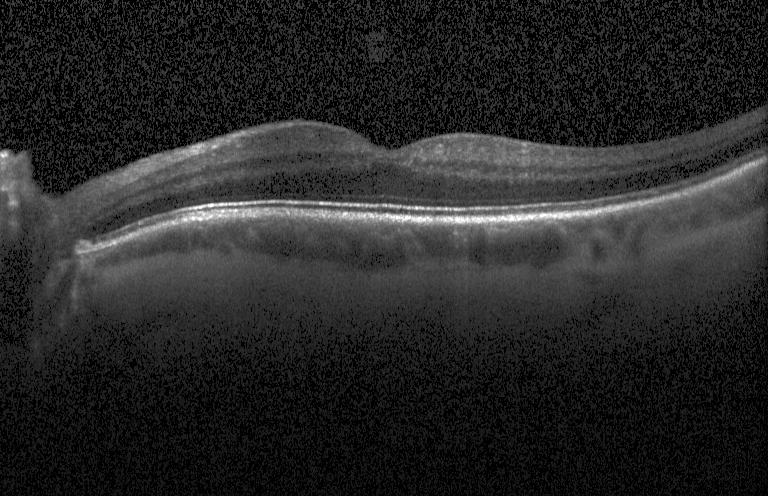 Impression: neither choroidal neovascularization, diabetic macular edema, nor drusen.